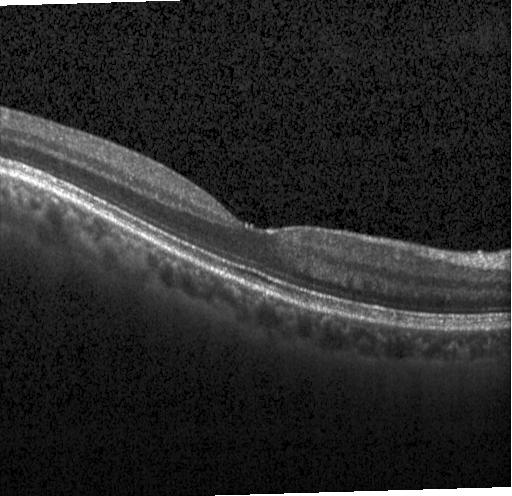

OCT scan showing no CNV, no DME, and no drusen.